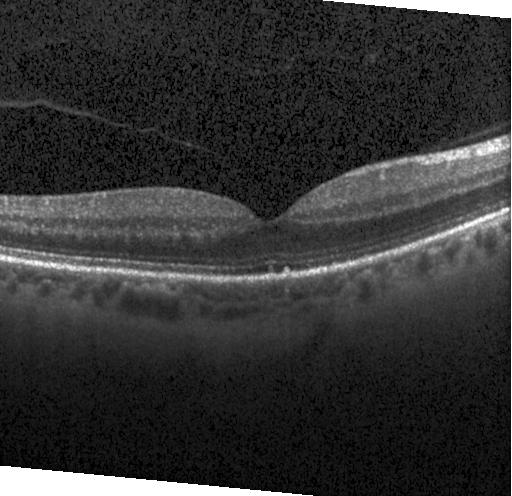

Retinal OCT cross-section. Spectral-domain OCT. The scan shows drusen.